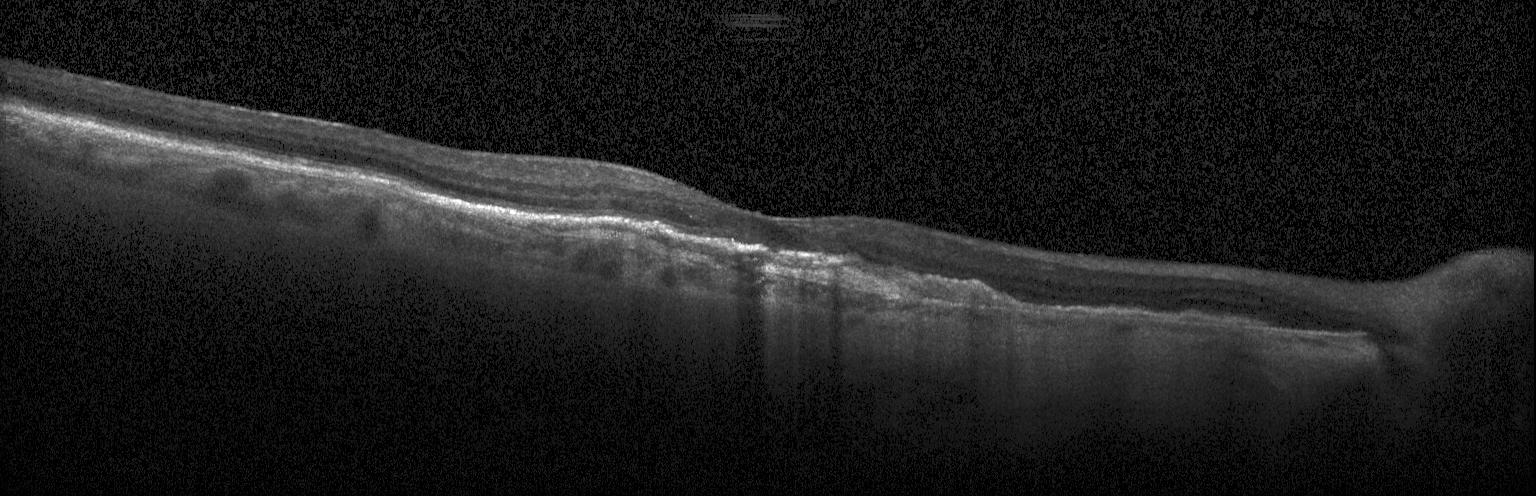

Retinal OCT B-scan · centered on the fovea · spectral-domain OCT · Heidelberg Spectralis.
Finding: a choroidal neovascular membrane.